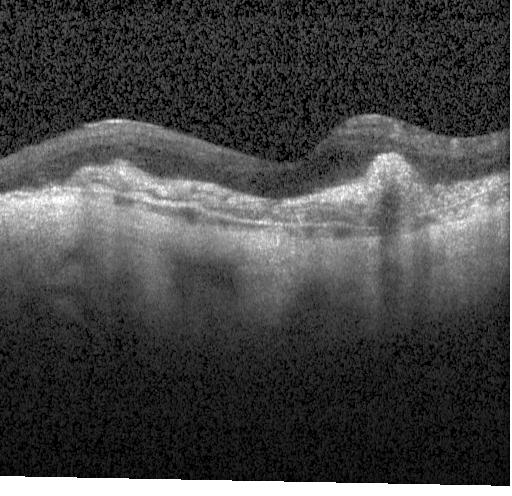 A choroidal neovascular membrane.